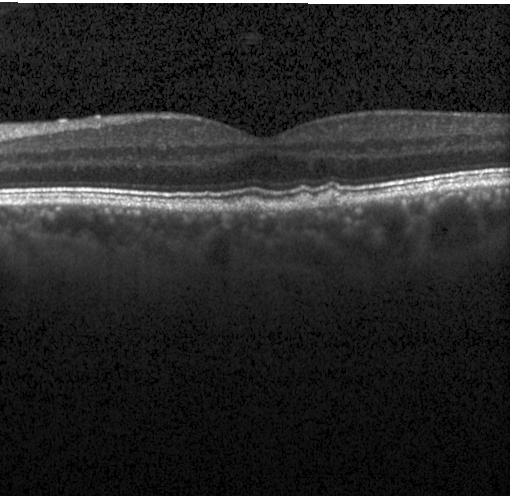
OCT line scan; spectral-domain optical coherence tomography; horizontal scan through the fovea; Heidelberg Spectralis OCT system.
Finding: multiple drusen.